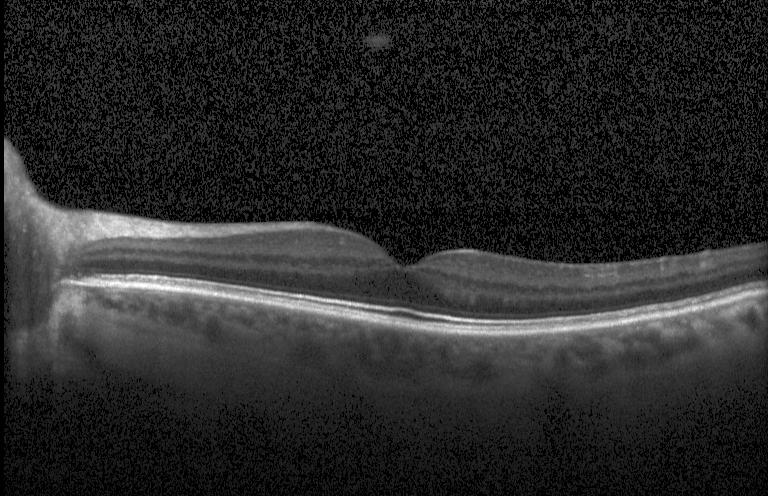
Diagnosis: no choroidal neovascularization, no diabetic macular edema, and no drusen.